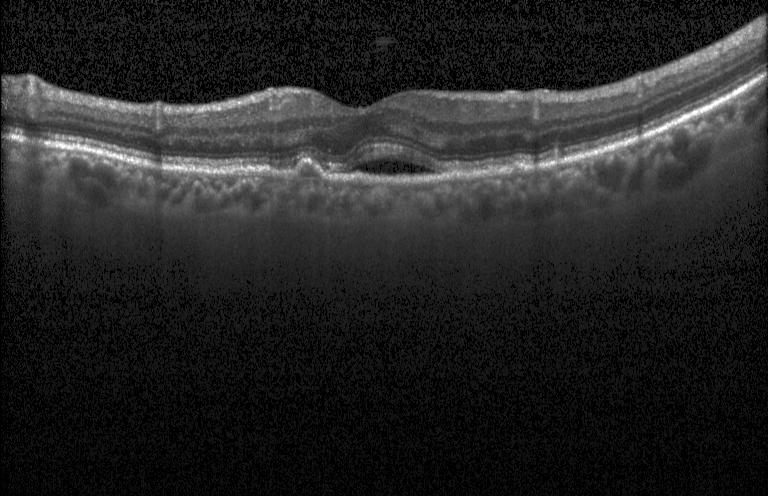
Optical coherence tomography B-scan.
Impression: choroidal neovascularization (CNV).